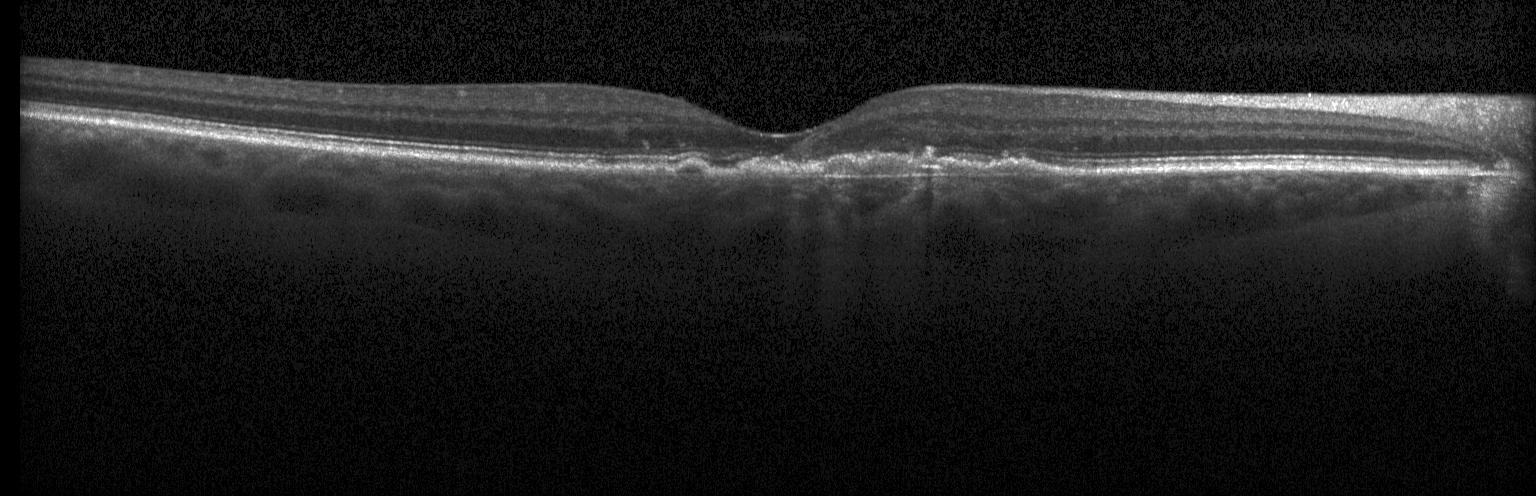

Heidelberg Spectralis; centered on the fovea; OCT B-scan
A choroidal neovascular membrane.